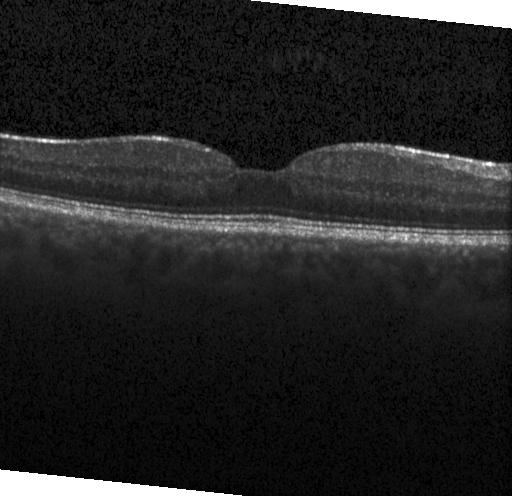

Retinal OCT cross-section, Heidelberg Spectralis. Finding: neither choroidal neovascularization, diabetic macular edema, nor drusen.